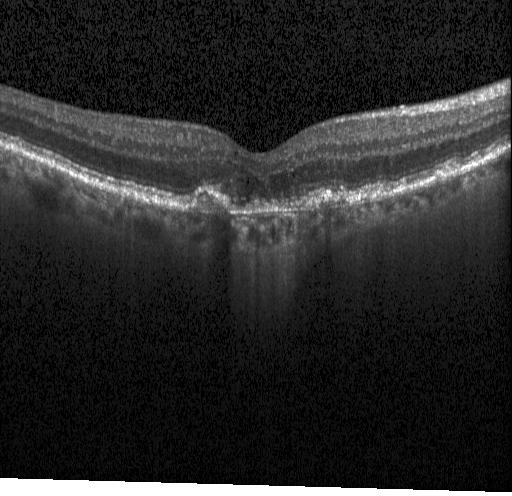 Centered on the fovea. Heidelberg Spectralis OCT system. Optical coherence tomography B-scan. Spectral-domain optical coherence tomography.
Impression: choroidal neovascularization.